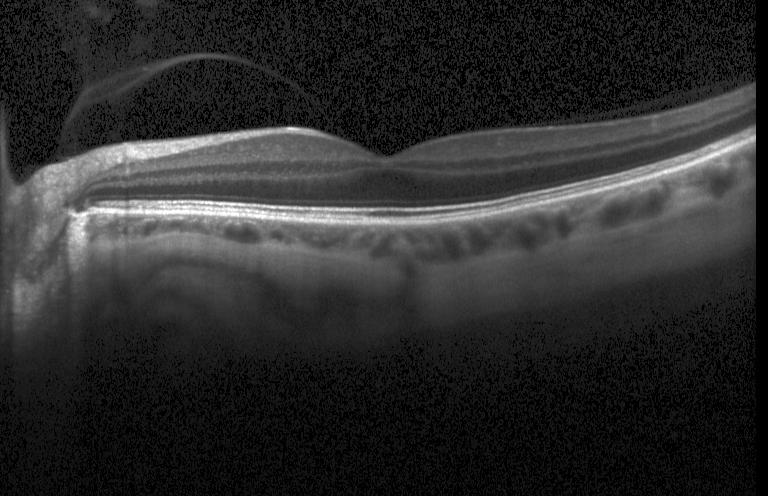 Spectral-domain OCT B-scan: no choroidal neovascularization, diabetic macular edema, or drusen.